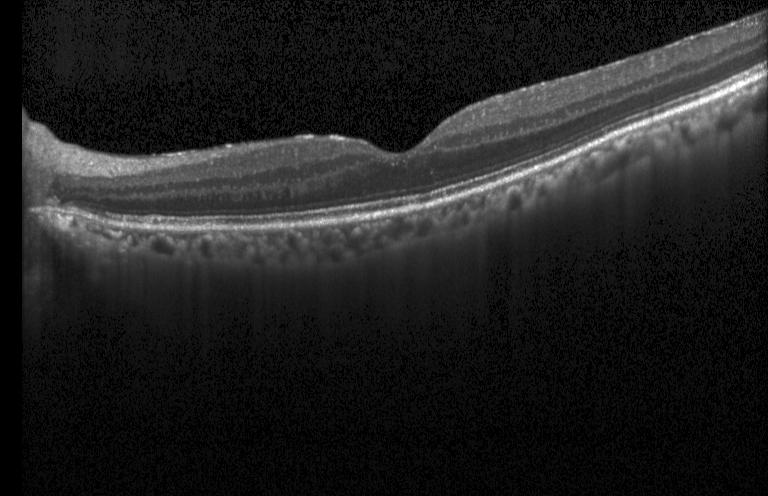 Macular scan; OCT B-scan; Heidelberg Spectralis OCT system — Diagnosis: neither CNV, DME, nor drusen.